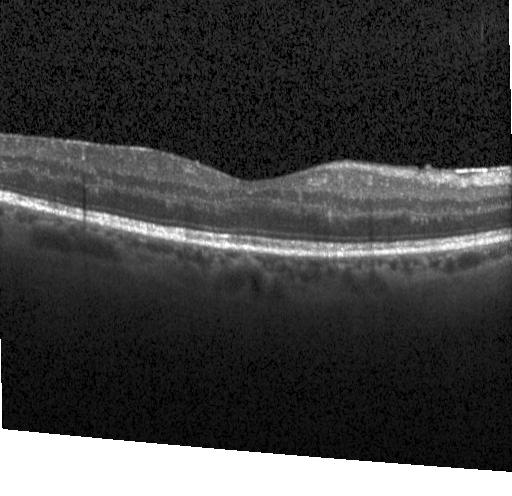 Macular OCT demonstrating no CNV, no DME, and no drusen.